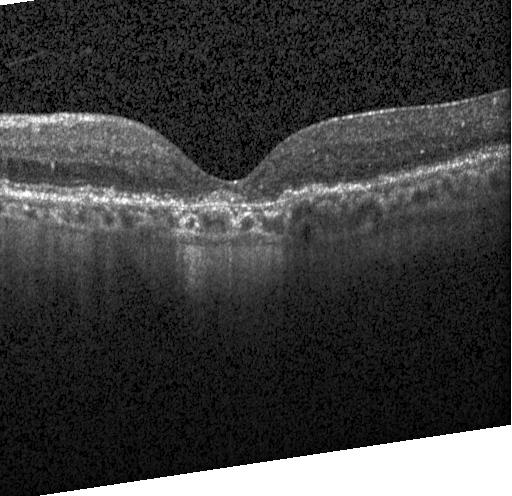
Finding: a choroidal neovascular membrane.